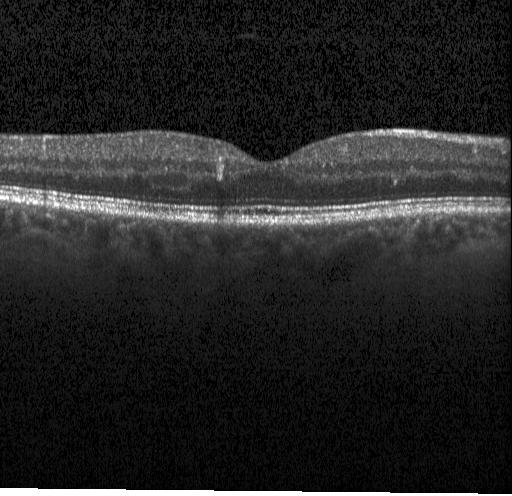 Acquired on a Heidelberg Spectralis; OCT line scan; spectral-domain optical coherence tomography
Macular OCT: no evidence of choroidal neovascularization, diabetic macular edema, or drusen.